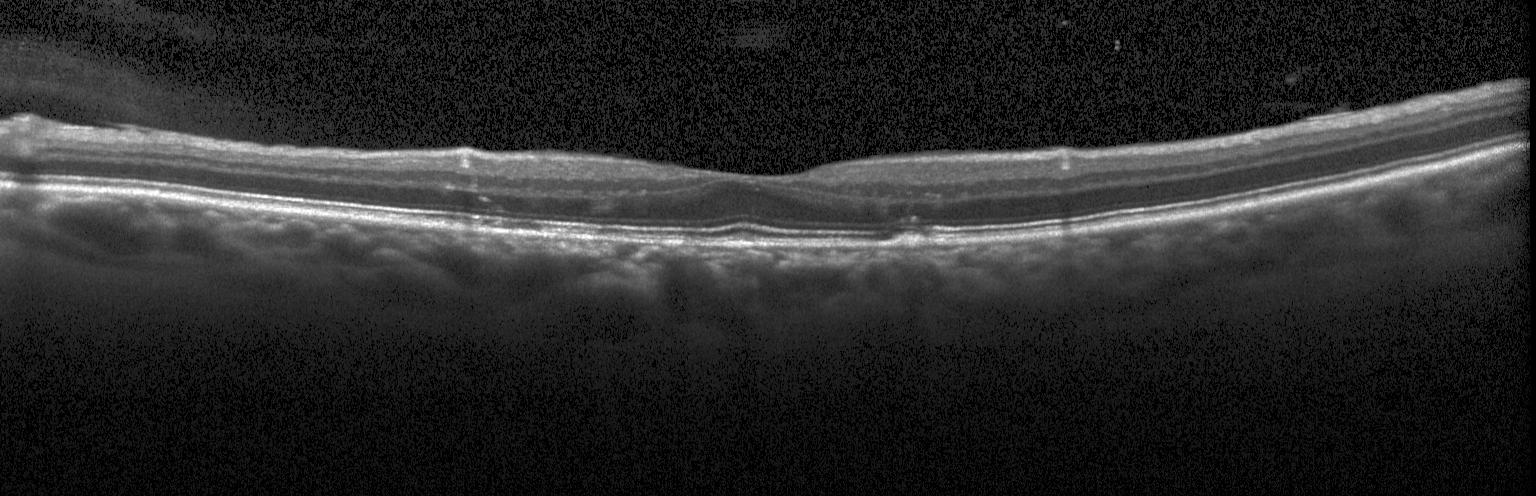

SD-OCT; OCT line scan. Sub-RPE drusenoid deposits.